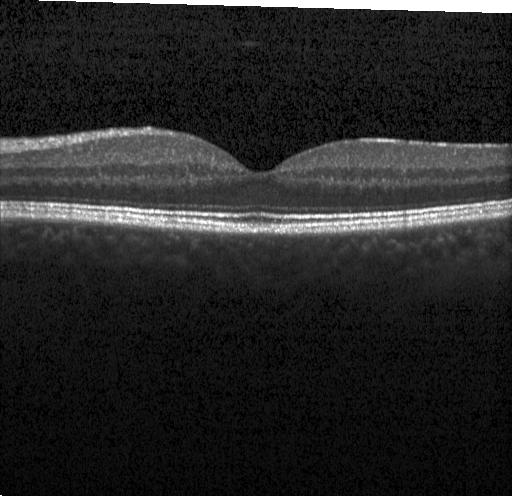

Retinal OCT B-scan; through the macula. Diagnosis: neither CNV, DME, nor drusen.